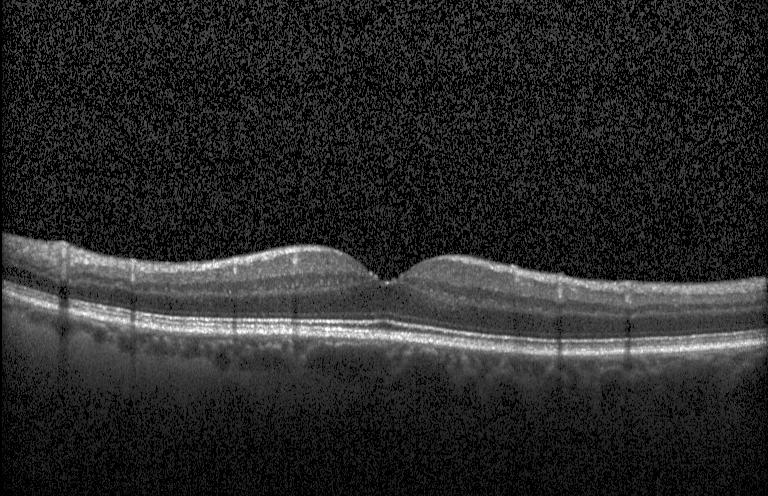 OCT line scan. Heidelberg Spectralis OCT system. SD-OCT. Fovea-centered
No choroidal neovascularization, diabetic macular edema, or drusen.